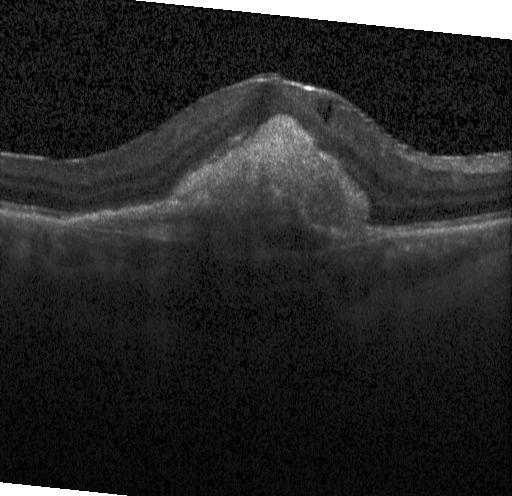 OCT B-scan. Macular OCT: choroidal neovascularization (CNV).